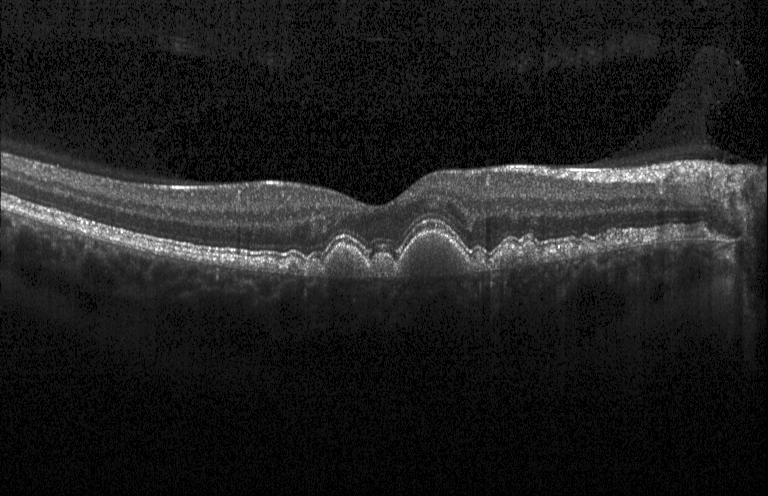 The scan shows sub-RPE drusenoid deposits.